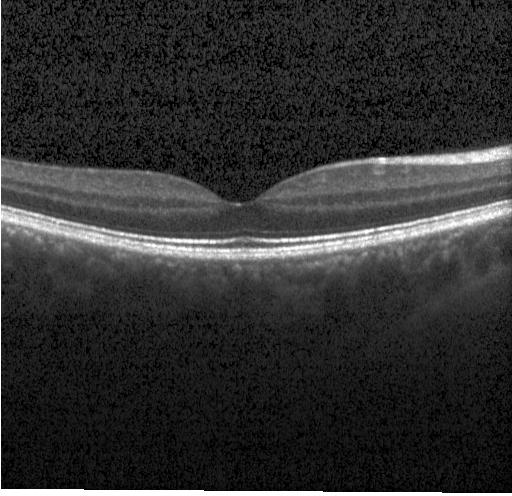

Retinal OCT cross-section — Finding: no choroidal neovascularization, diabetic macular edema, or drusen.